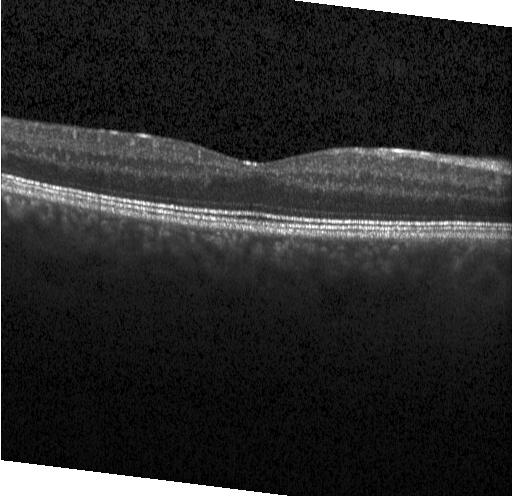 Spectral-domain OCT. Instrument: Heidelberg Spectralis. Optical coherence tomography scan. Horizontal scan through the fovea — This B-scan demonstrates neither choroidal neovascularization, diabetic macular edema, nor drusen.